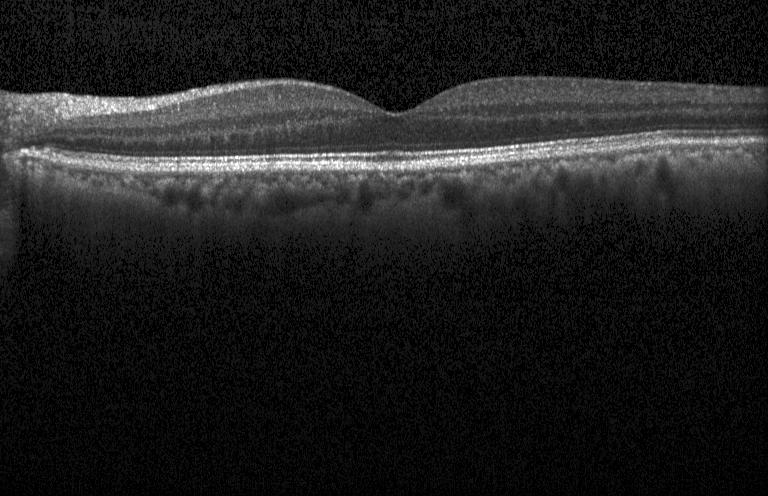
Diagnosis: neither choroidal neovascularization, diabetic macular edema, nor drusen.